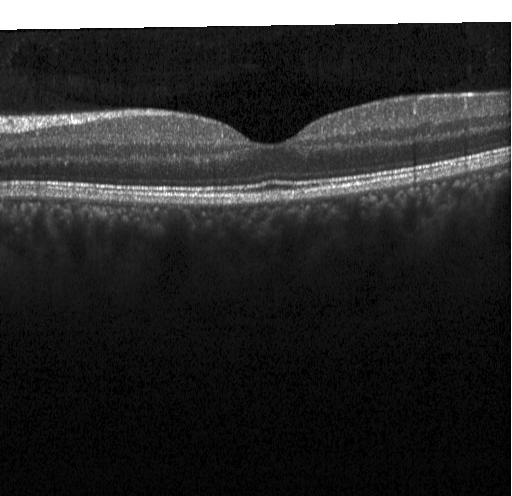
The scan shows no CNV, DME, or drusen.